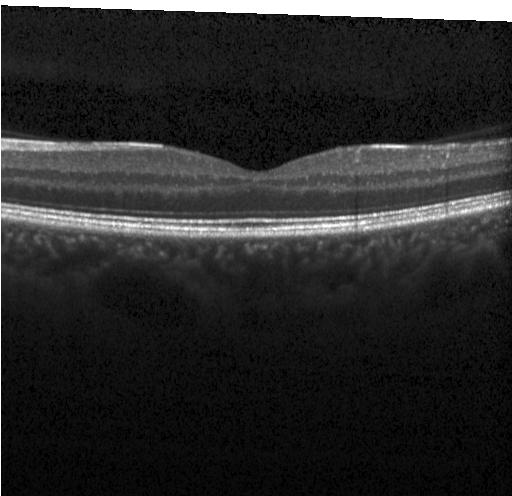

Centered on the fovea, optical coherence tomography B-scan, instrument: Heidelberg Spectralis. Impression: neither CNV, DME, nor drusen.